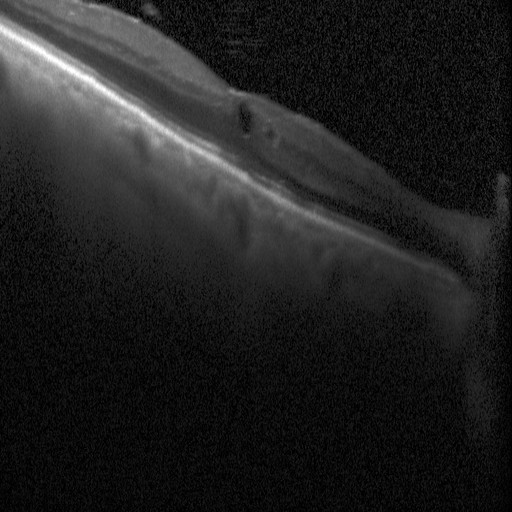
SD-OCT, OCT B-scan — Assessment: diabetic macular edema.